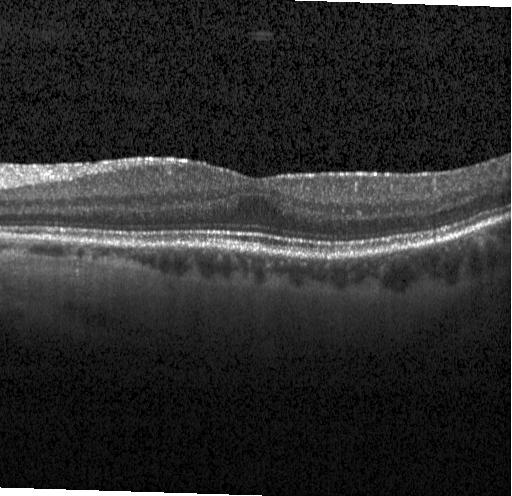 Impression: no CNV, no DME, and no drusen.